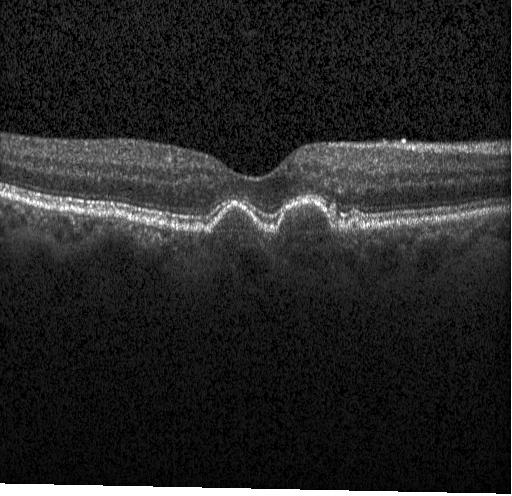 Impression: multiple drusen.